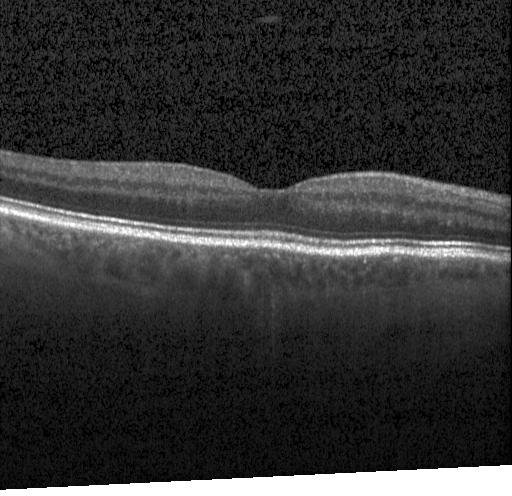 Macular OCT: no choroidal neovascularization, no diabetic macular edema, and no drusen.